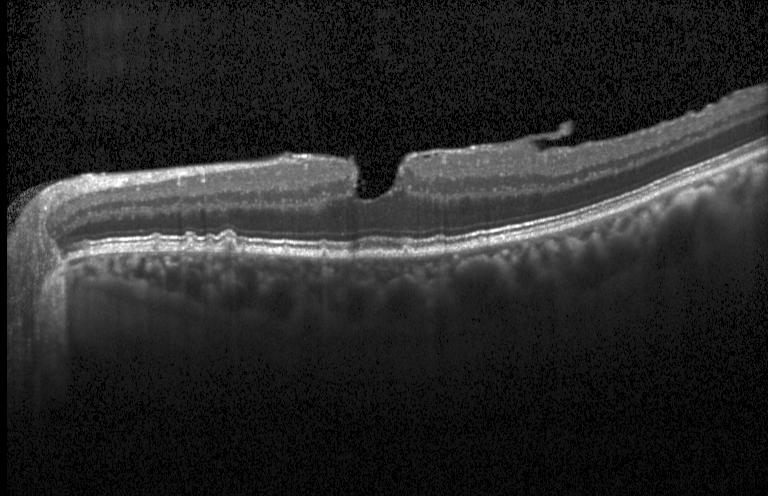 Instrument: Heidelberg Spectralis. SD-OCT. Retinal OCT B-scan — This B-scan demonstrates sub-RPE drusenoid deposits.